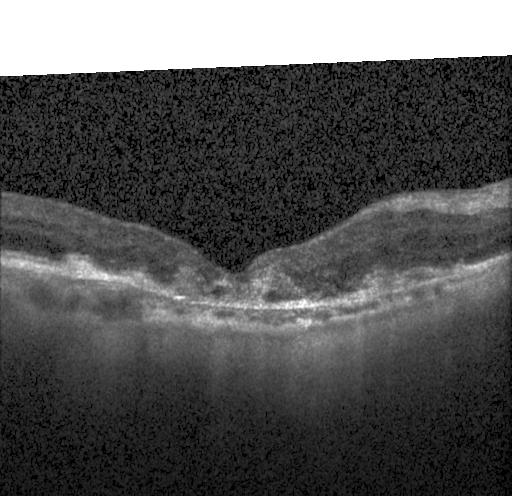

Retinal OCT cross-section; macular scan; acquired on a Heidelberg Spectralis. OCT finding: a choroidal neovascular membrane.